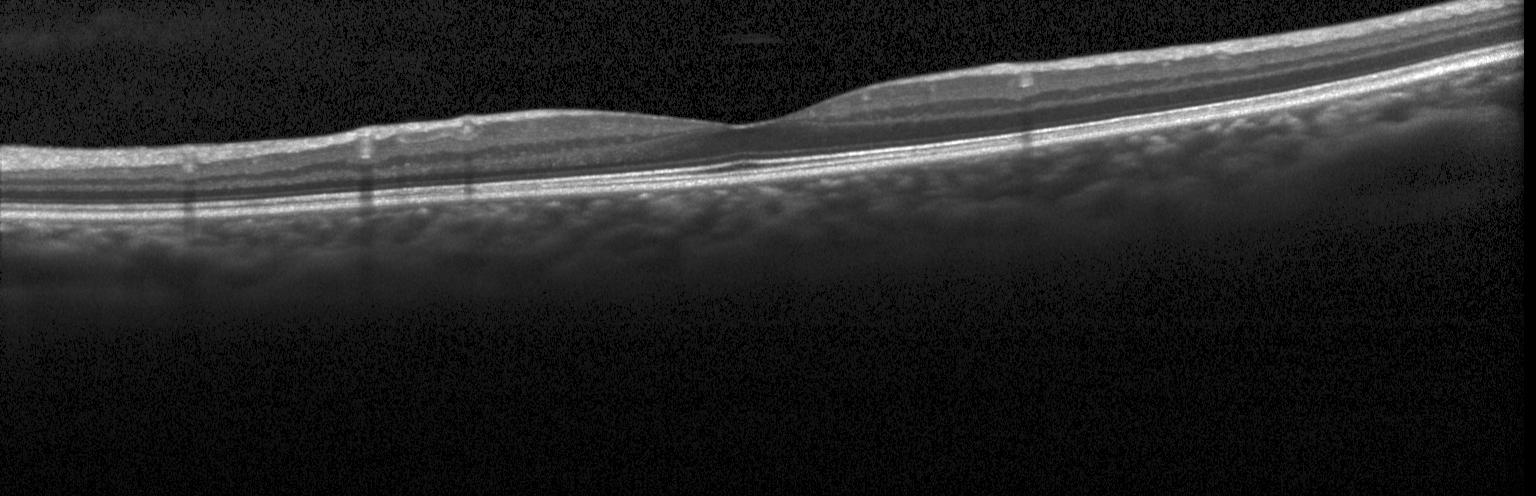

Instrument: Heidelberg Spectralis; centered on the fovea; retinal OCT cross-section; spectral-domain optical coherence tomography
Finding: no CNV, DME, or drusen.